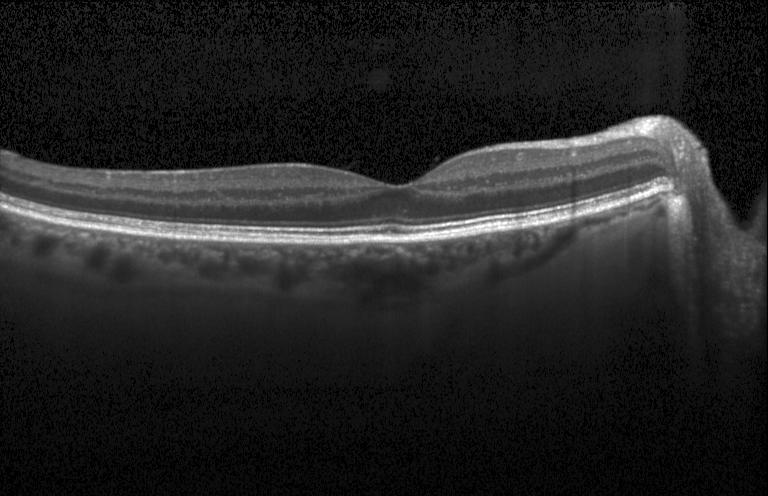
Diagnosis: no choroidal neovascularization, diabetic macular edema, or drusen.